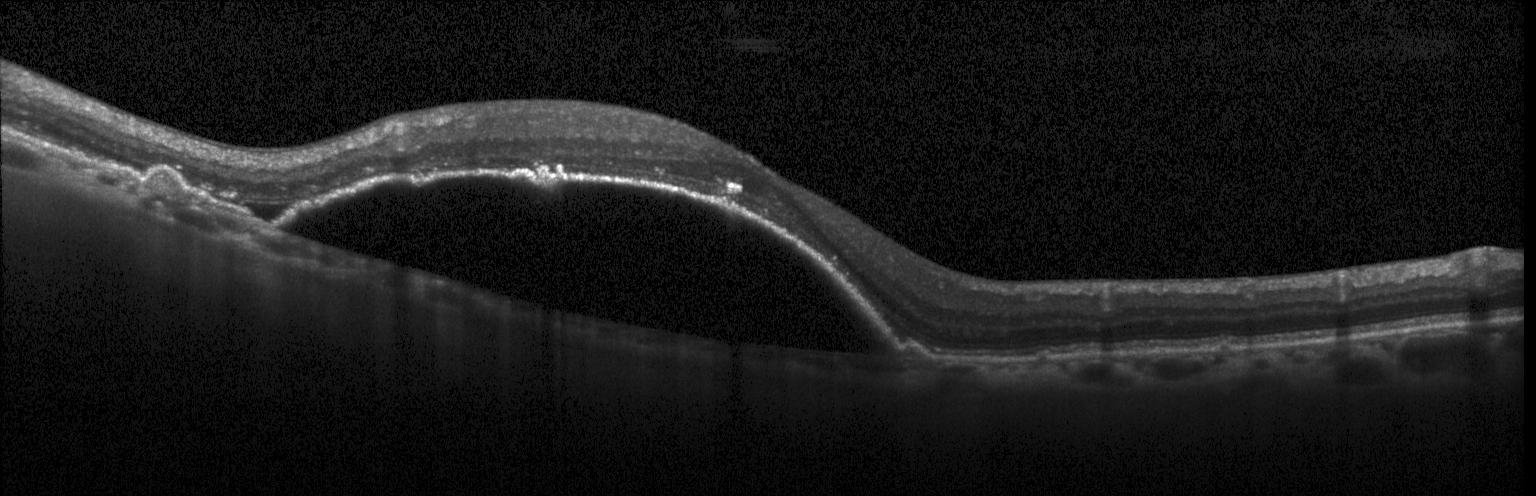 Assessment: CNV.